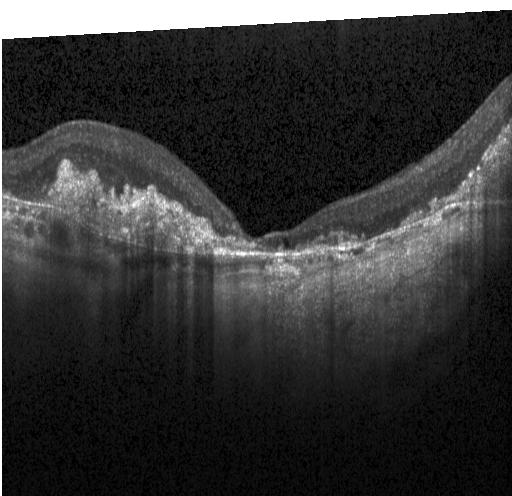
Horizontal scan through the fovea; SD-OCT; OCT line scan; Heidelberg Spectralis.
Assessment: choroidal neovascularization.